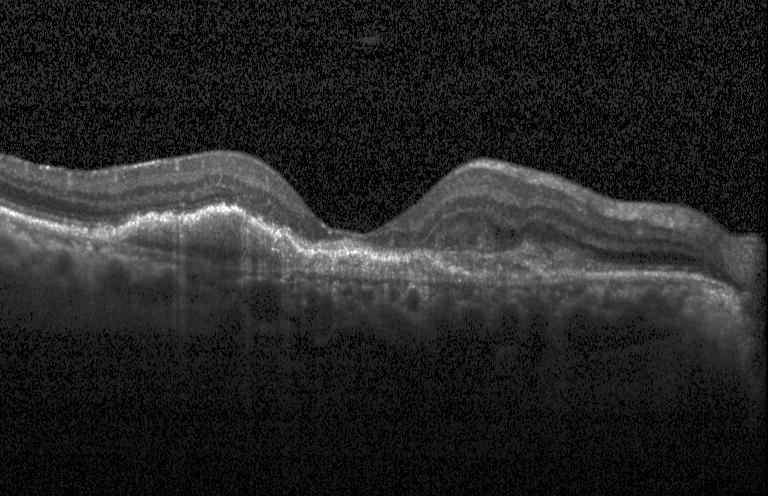 This B-scan demonstrates a choroidal neovascular membrane.